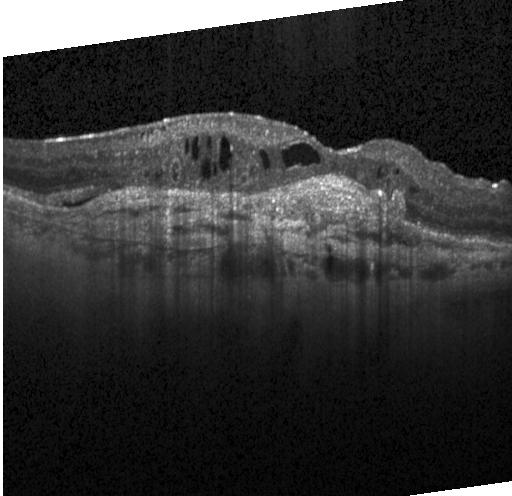
Macular OCT demonstrating choroidal neovascularization.